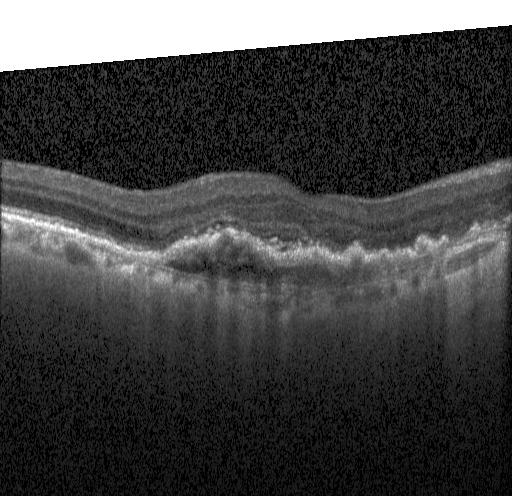 Finding: a choroidal neovascular membrane.